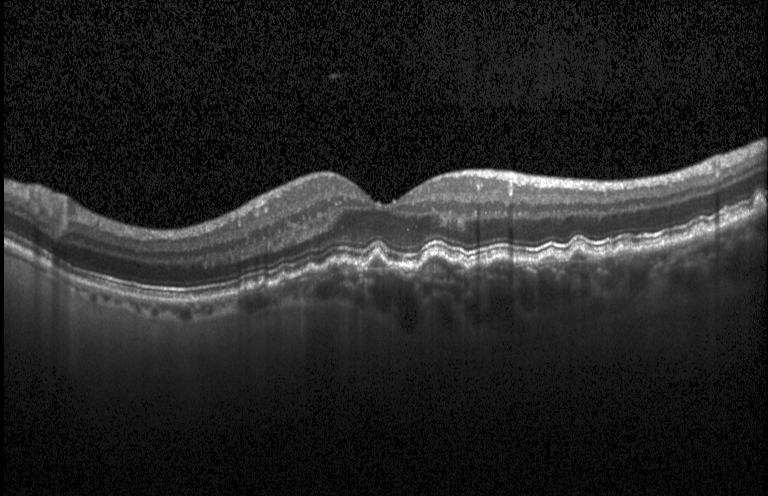

Acquired on a Heidelberg Spectralis. OCT line scan. Impression: multiple drusen.